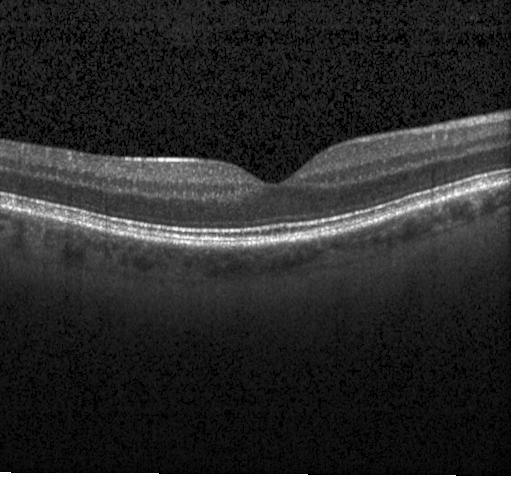
OCT B-scan — Assessment: no choroidal neovascularization, diabetic macular edema, or drusen.